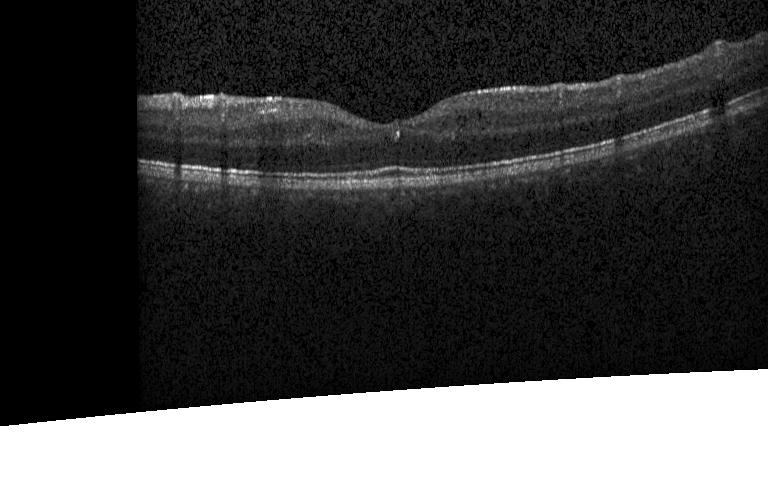

Retinal OCT cross-section
Diagnosis: diabetic macular edema (DME).